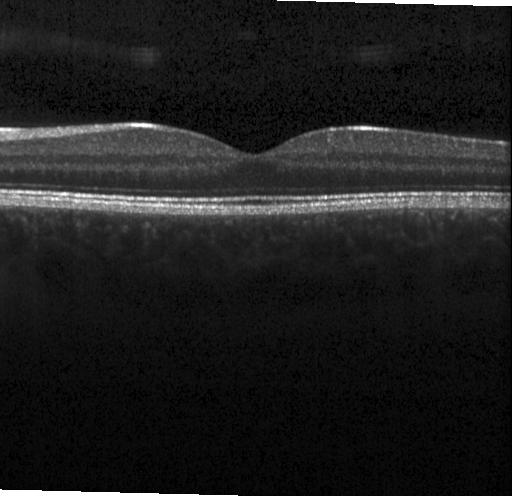

OCT B-scan — Impression: no choroidal neovascularization, diabetic macular edema, or drusen.